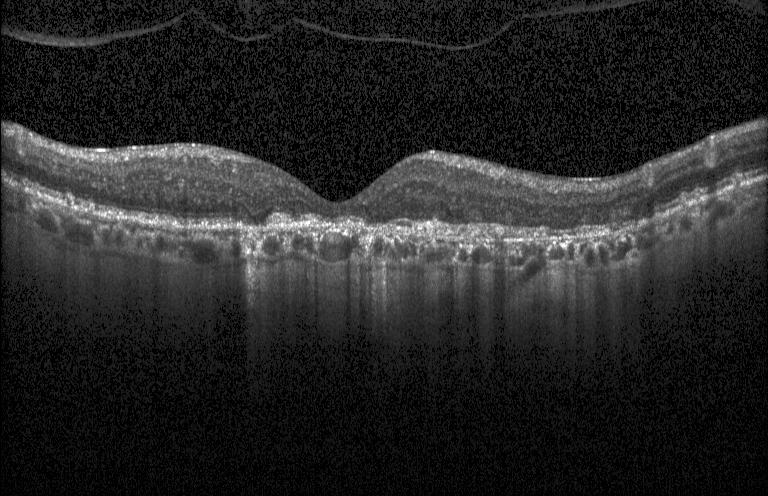
Spectral-domain optical coherence tomography. OCT line scan
Impression: choroidal neovascularization (CNV).